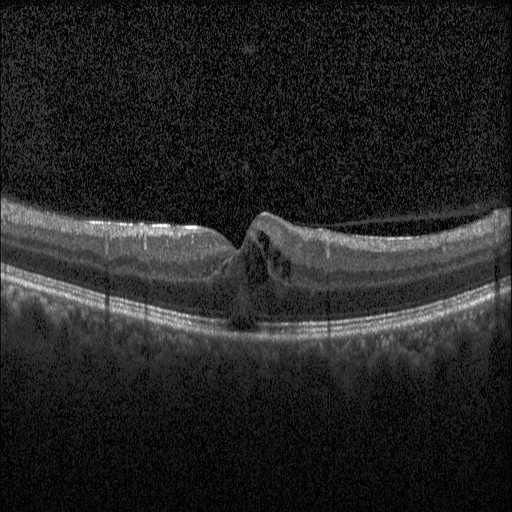

Optical coherence tomography B-scan. Diagnosis: diabetic macular edema (DME).